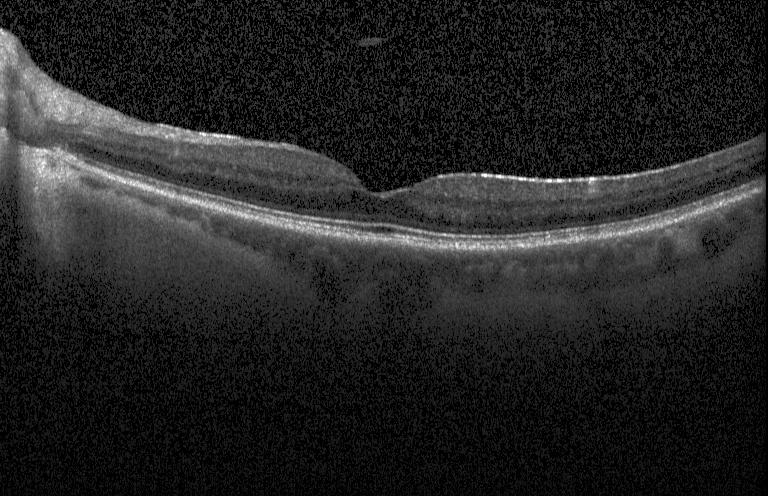 OCT line scan.
Macular OCT: neither choroidal neovascularization, diabetic macular edema, nor drusen.